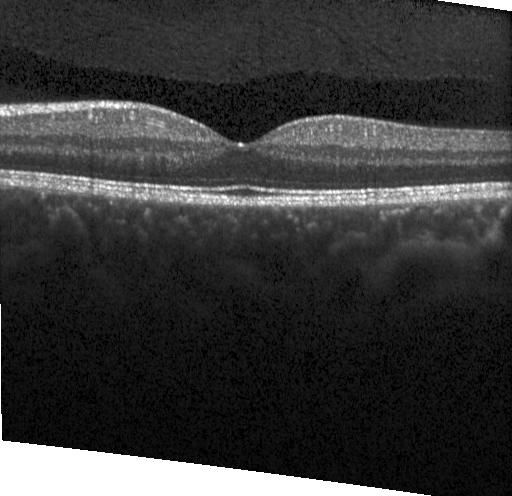

Neither choroidal neovascularization, diabetic macular edema, nor drusen.